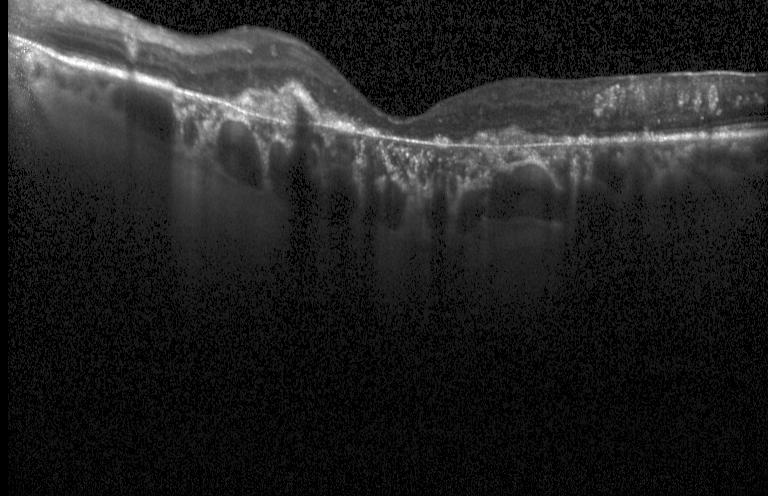
OCT finding: a choroidal neovascular membrane.